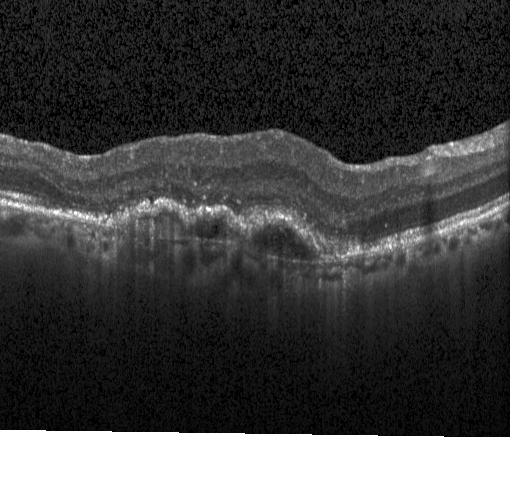 SD-OCT · retinal OCT B-scan
CNV.